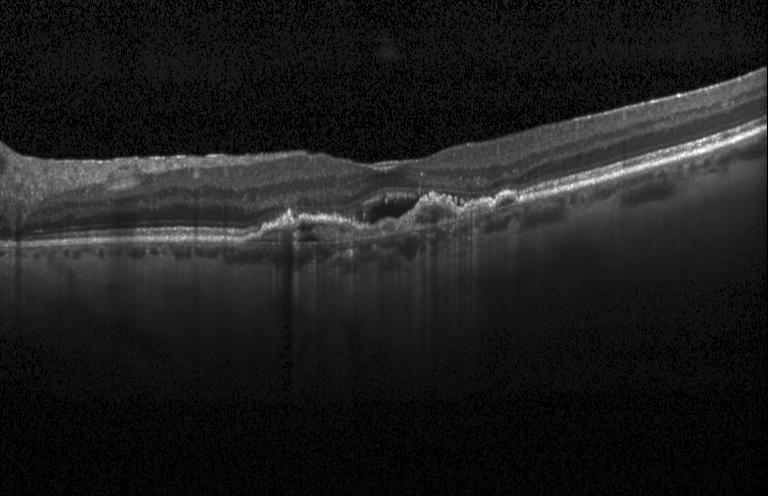 OCT finding: a choroidal neovascular membrane.